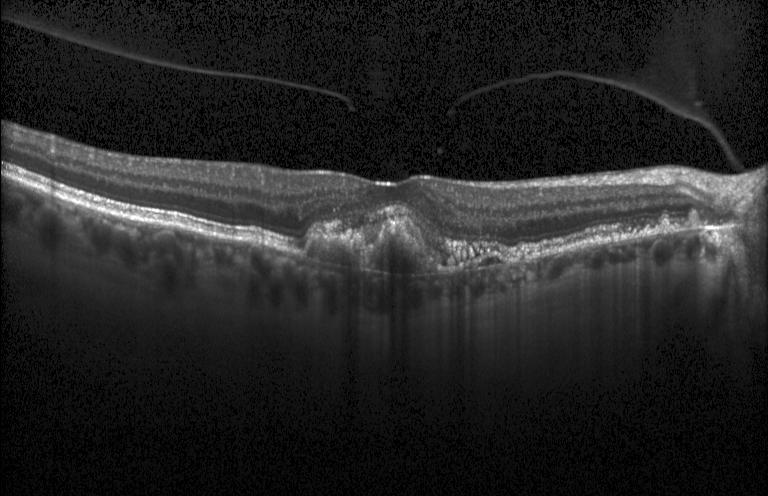 Spectral-domain optical coherence tomography · instrument: Heidelberg Spectralis · retinal OCT cross-section. Finding: a choroidal neovascular membrane.